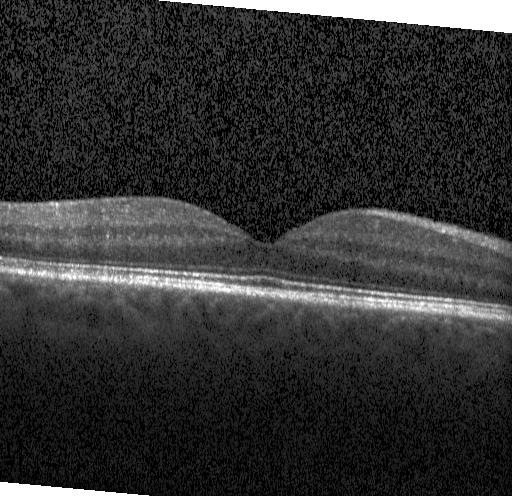

Optical coherence tomography B-scan; spectral-domain OCT. Diagnosis: no evidence of CNV, DME, or drusen.